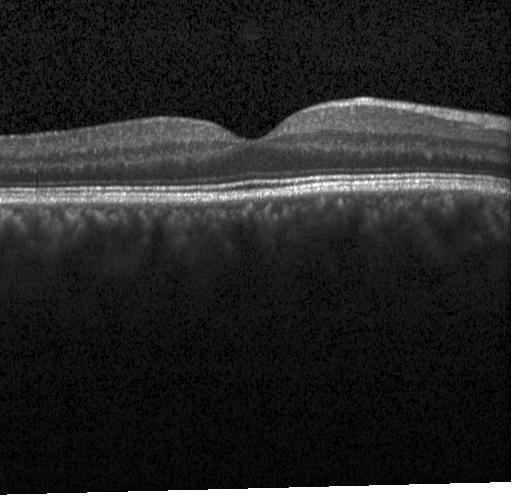 Spectral-domain OCT B-scan: neither choroidal neovascularization, diabetic macular edema, nor drusen.